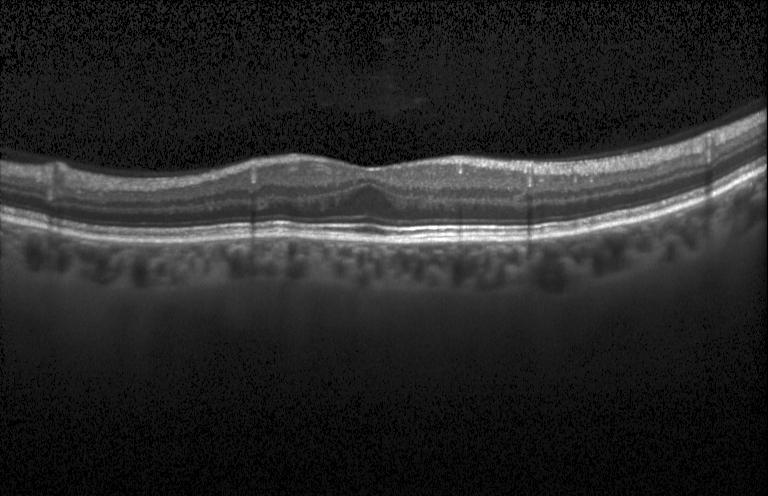 Diagnosis: no choroidal neovascularization, diabetic macular edema, or drusen.